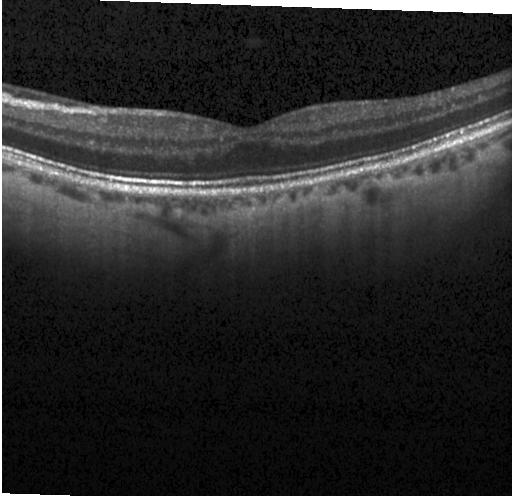 Macular OCT demonstrating no evidence of choroidal neovascularization, diabetic macular edema, or drusen.